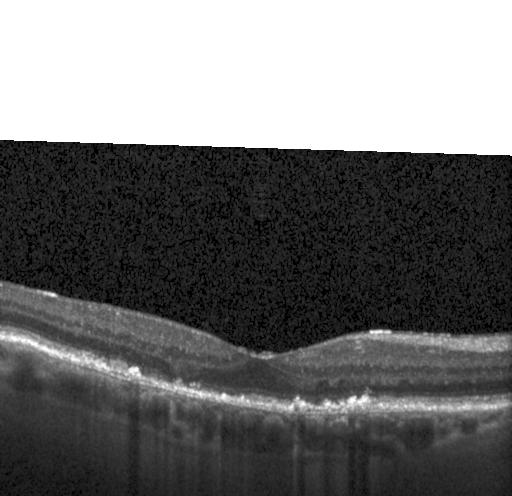 OCT line scan. Impression: multiple drusen.